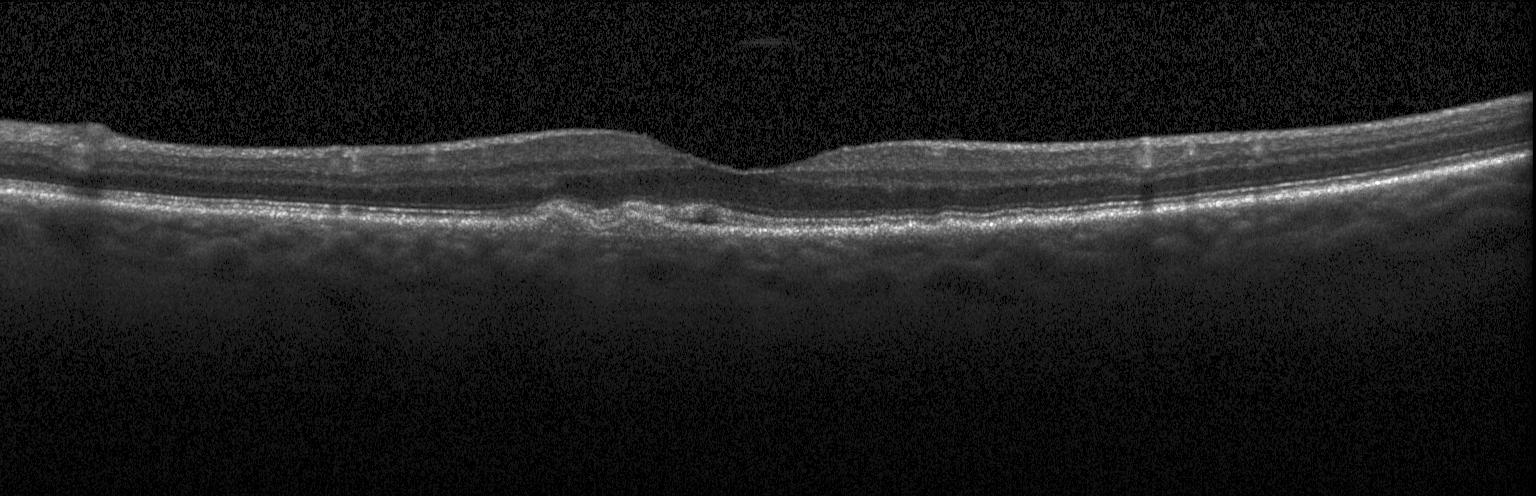

Spectral-domain OCT B-scan: a choroidal neovascular membrane.